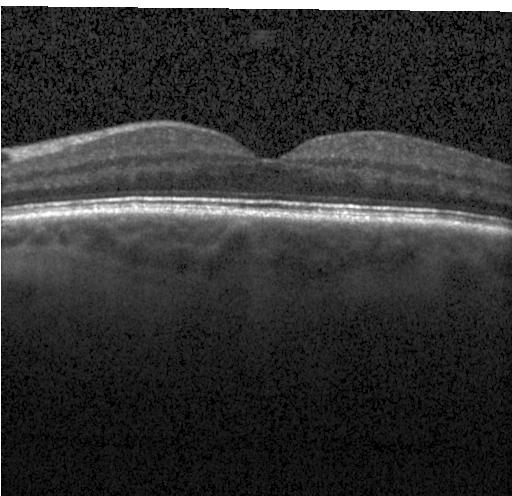
Impression: no evidence of choroidal neovascularization, diabetic macular edema, or drusen.